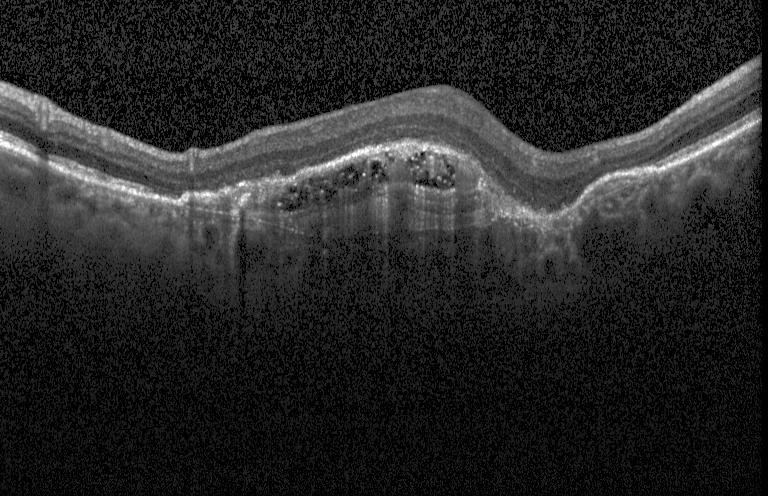
Macular OCT: choroidal neovascularization (CNV).